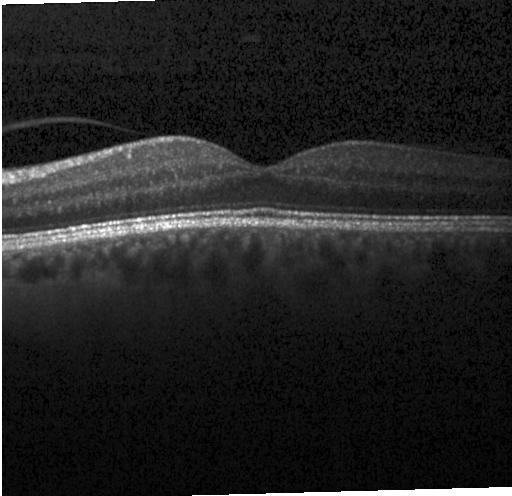 Spectral-domain optical coherence tomography, OCT line scan.
Dx: no CNV, no DME, and no drusen.